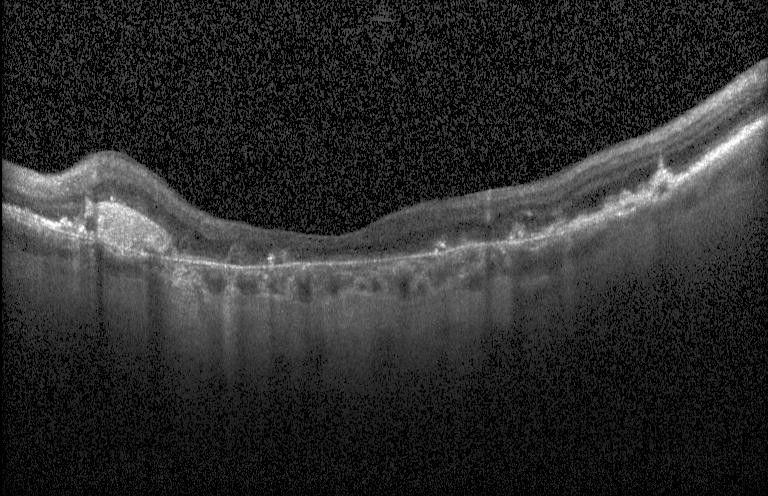
Centered on the fovea; optical coherence tomography scan; spectral-domain optical coherence tomography; Heidelberg Spectralis OCT system — This B-scan demonstrates a choroidal neovascular membrane.